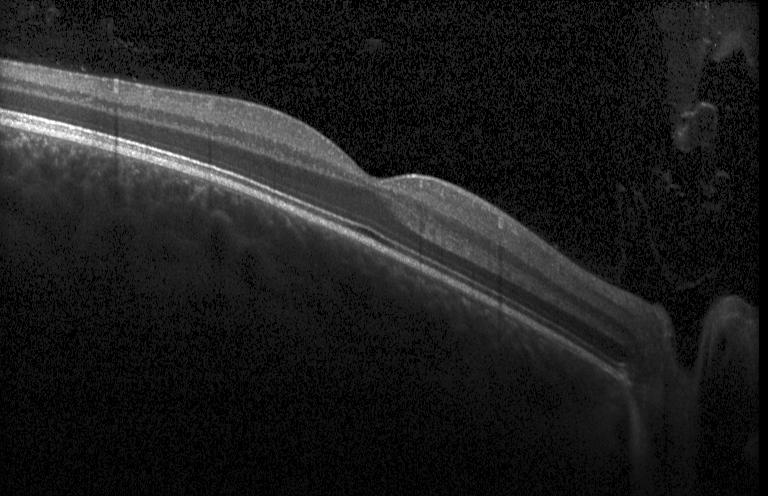 This B-scan demonstrates neither choroidal neovascularization, diabetic macular edema, nor drusen.